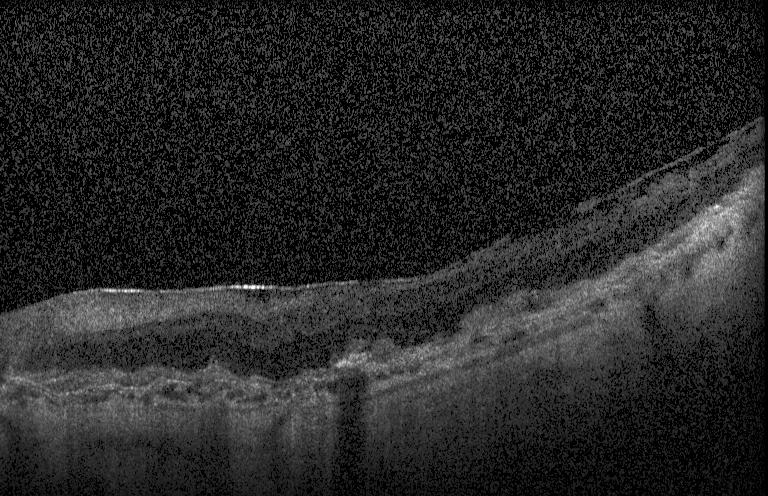

OCT scan showing a choroidal neovascular membrane.